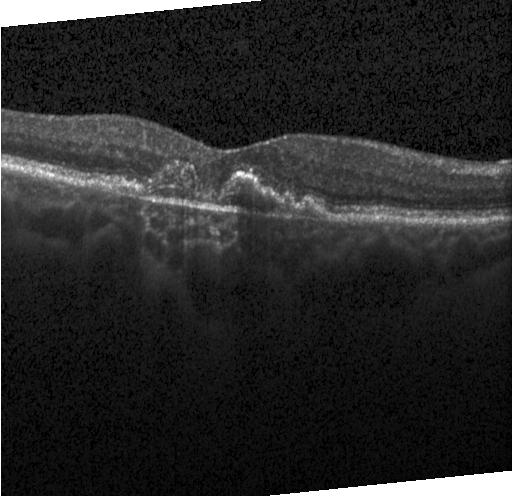

Heidelberg Spectralis OCT system, SD-OCT, optical coherence tomography scan, centered on the fovea
Diagnosis: a choroidal neovascular membrane.